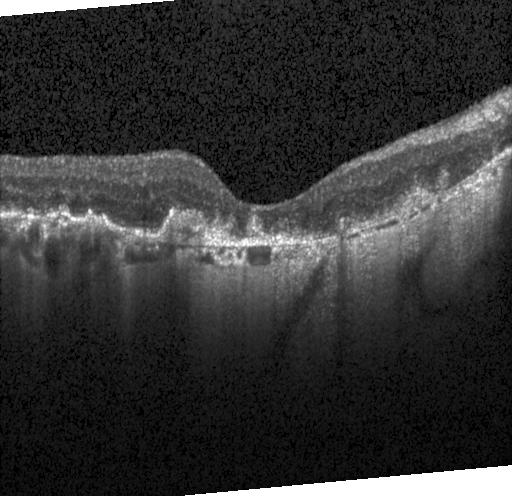 Diagnosis: a choroidal neovascular membrane.